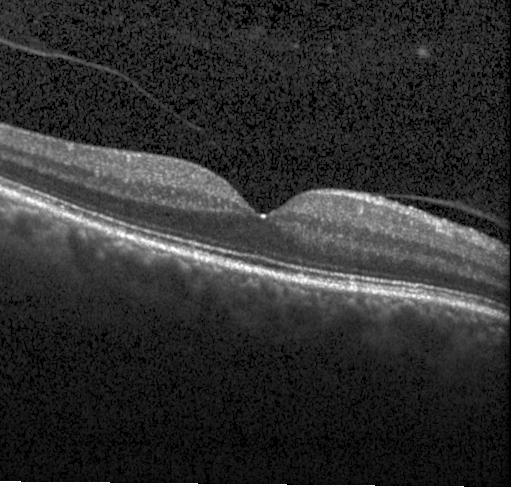

Fovea-centered. Spectral-domain optical coherence tomography. Retinal OCT cross-section. Finding: no evidence of CNV, DME, or drusen.